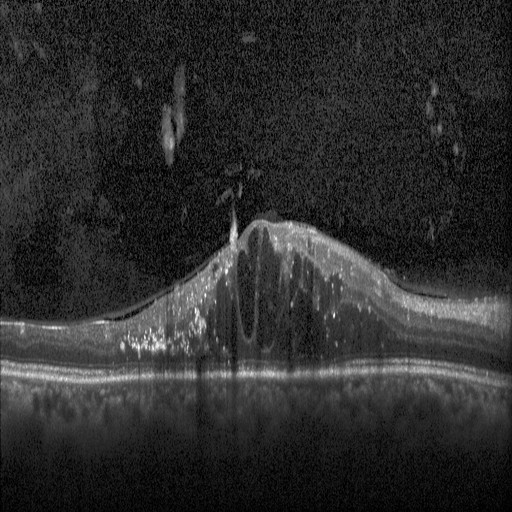 Optical coherence tomography B-scan · Heidelberg Spectralis. Impression: diabetic macular edema (DME).